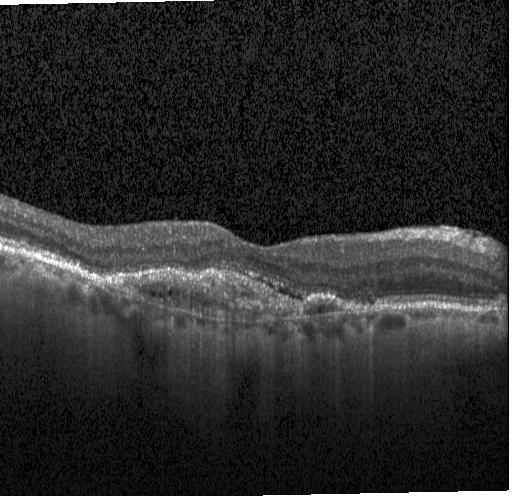
Impression: a choroidal neovascular membrane.